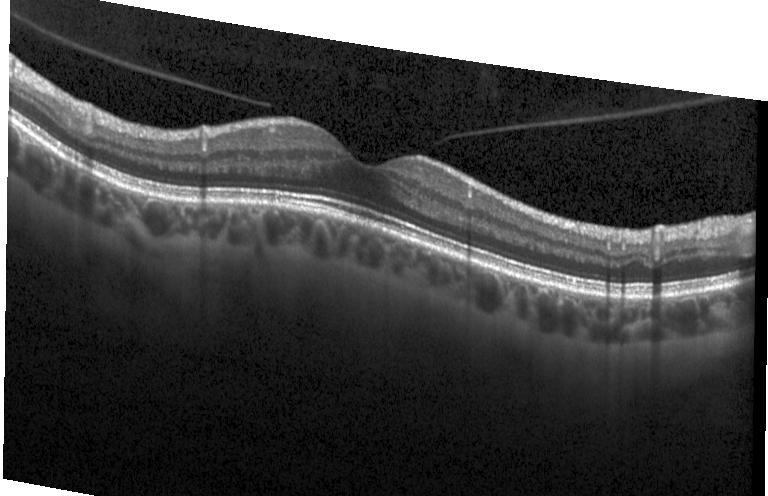 OCT B-scan showing neither CNV, DME, nor drusen.